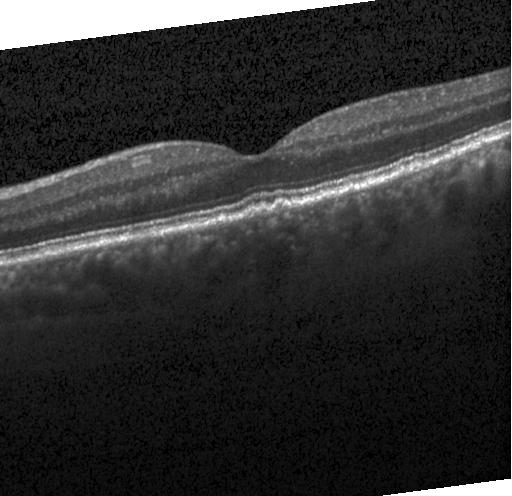 Optical coherence tomography B-scan, acquired on a Heidelberg Spectralis, spectral-domain OCT, macular scan
This B-scan demonstrates drusen.